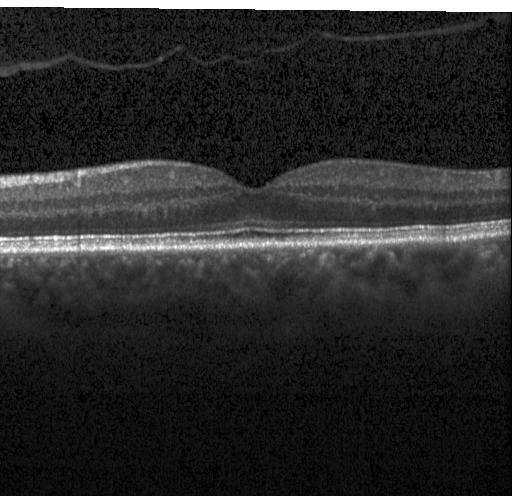
Dx: no choroidal neovascularization, diabetic macular edema, or drusen.